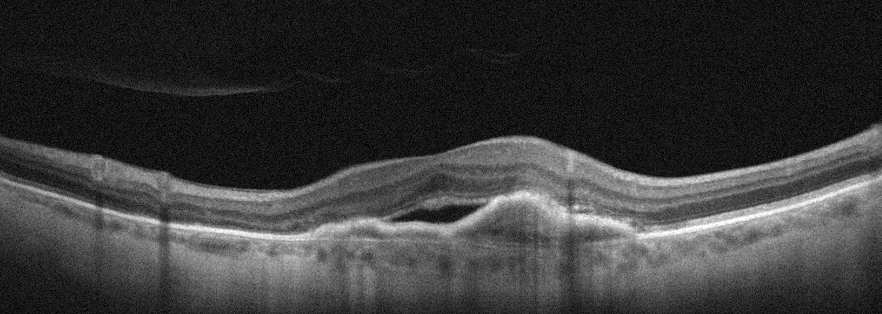
Oculus sinister · optical coherence tomography B-scan.
Impression: age-related macular degeneration (AMD).